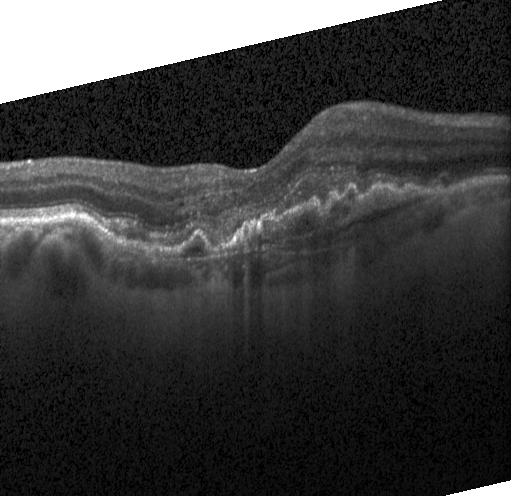 OCT B-scan showing CNV.